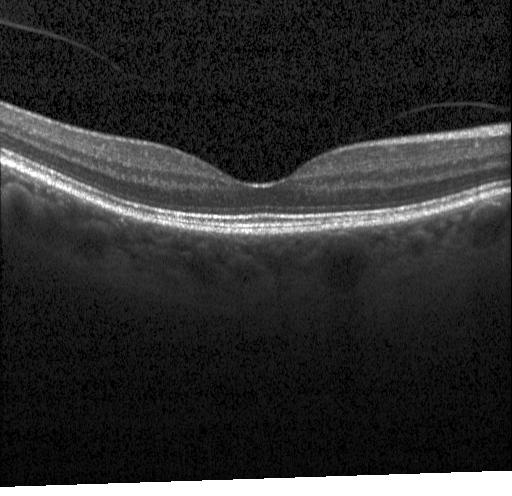
Through the macula · spectral-domain OCT · instrument: Heidelberg Spectralis · optical coherence tomography scan
Impression: neither choroidal neovascularization, diabetic macular edema, nor drusen.